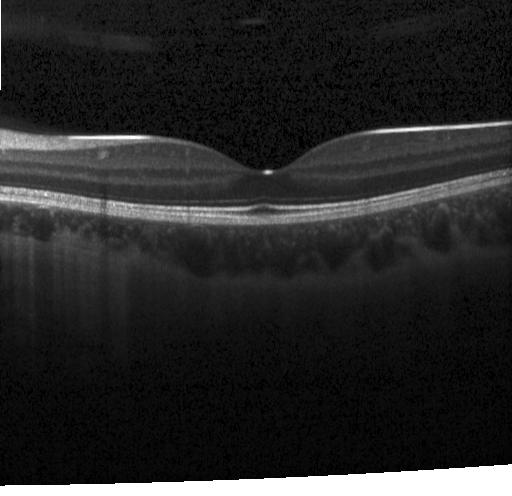

Spectral-domain optical coherence tomography; retinal OCT B-scan; fovea-centered; Heidelberg Spectralis OCT system.
Finding: no choroidal neovascularization, diabetic macular edema, or drusen.